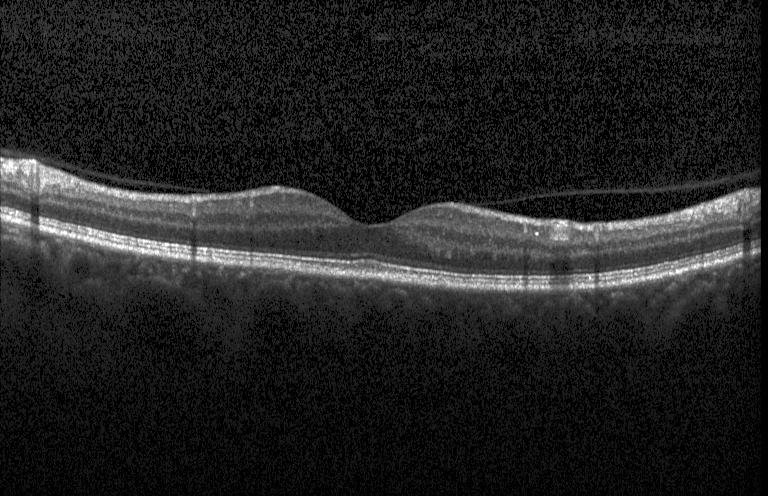
OCT line scan. Centered on the fovea. Heidelberg Spectralis. Diagnosis: no choroidal neovascularization, no diabetic macular edema, and no drusen.